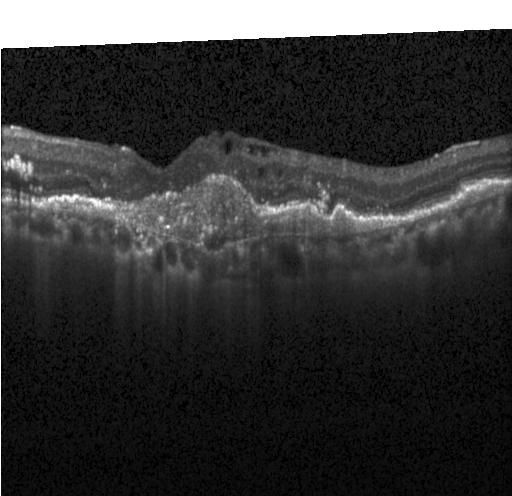 OCT B-scan, through the macula, spectral-domain OCT, Heidelberg Spectralis OCT system
CNV.